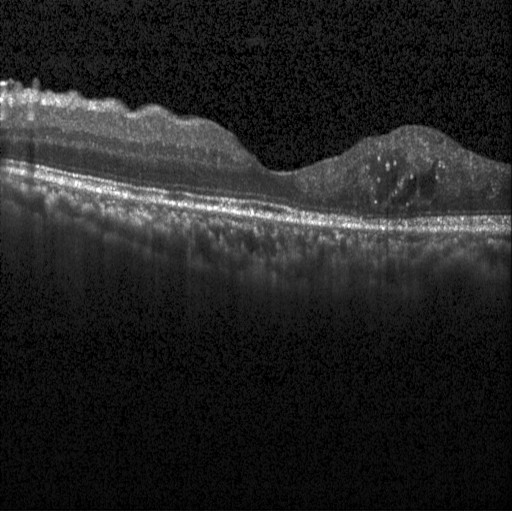
Instrument: Heidelberg Spectralis; fovea-centered; retinal OCT cross-section. Impression: DME.